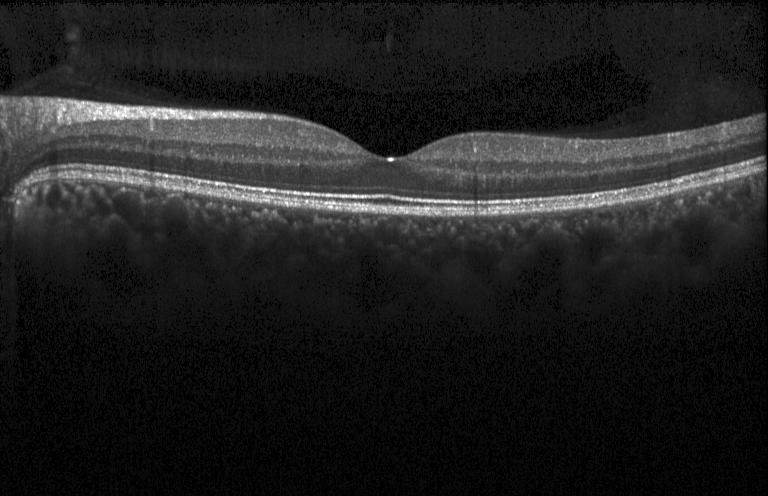

OCT B-scan; SD-OCT — Finding: no evidence of choroidal neovascularization, diabetic macular edema, or drusen.